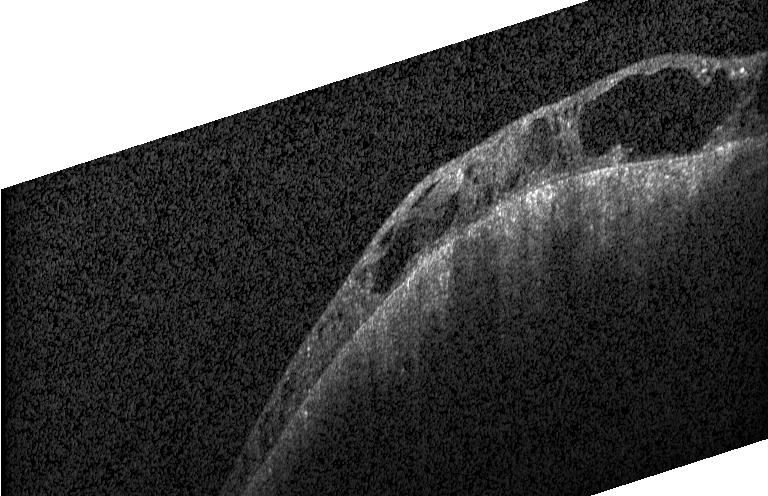 Optical coherence tomography B-scan.
Impression: diabetic macular edema.